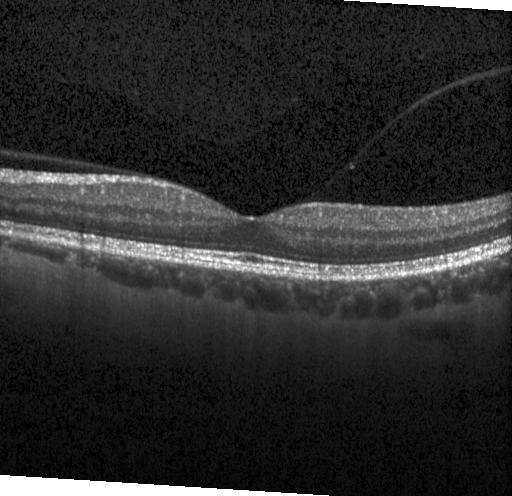
Spectral-domain OCT, optical coherence tomography scan. Diagnosis: no choroidal neovascularization, no diabetic macular edema, and no drusen.